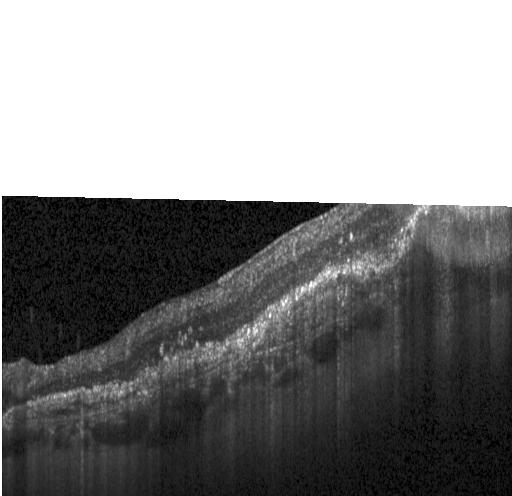
Macular OCT demonstrating choroidal neovascularization.